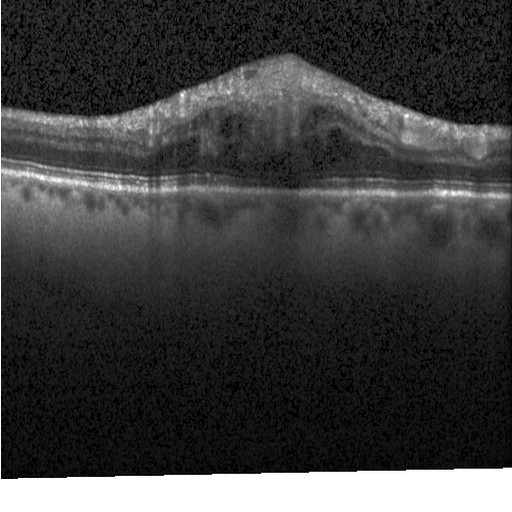

Retinal OCT B-scan. Diabetic macular edema.